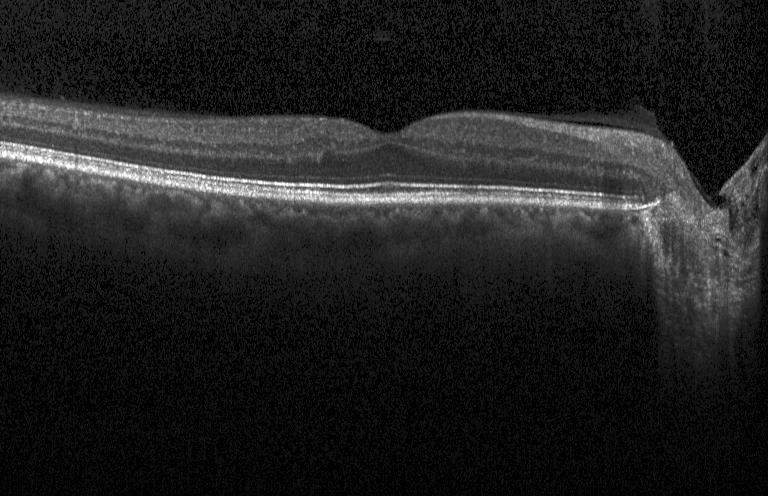
No CNV, no DME, and no drusen.